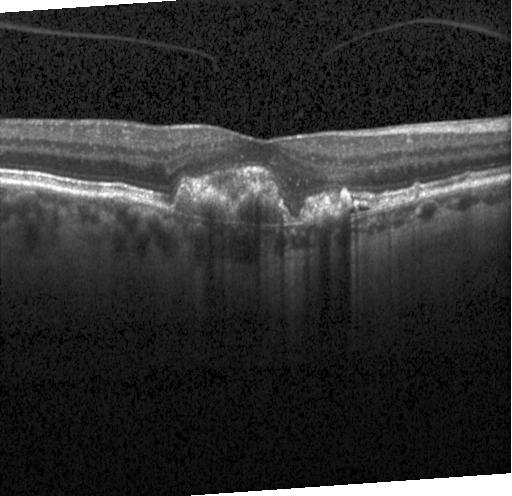
Optical coherence tomography B-scan. Through the macula. Macular OCT: a choroidal neovascular membrane.